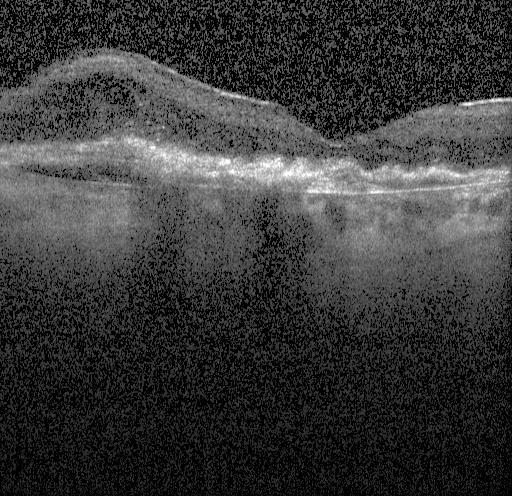
OCT line scan.
Impression: a choroidal neovascular membrane.